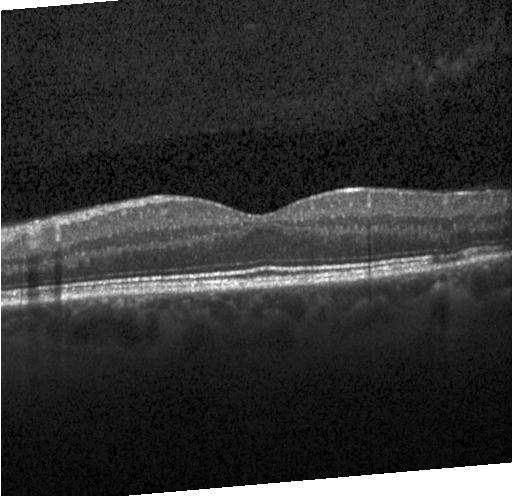
Instrument: Heidelberg Spectralis, spectral-domain optical coherence tomography, through the macula, optical coherence tomography B-scan
Dx: no evidence of choroidal neovascularization, diabetic macular edema, or drusen.